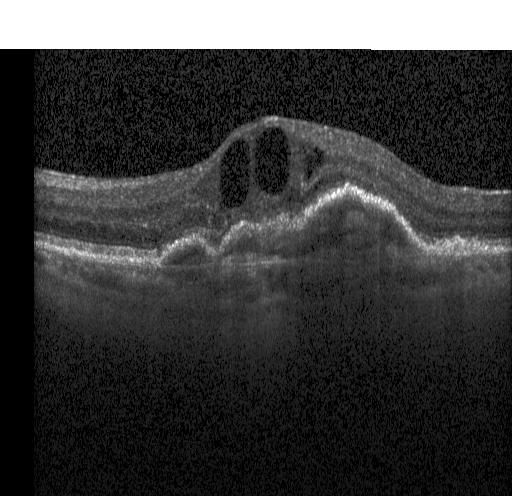

Finding: choroidal neovascularization (CNV).